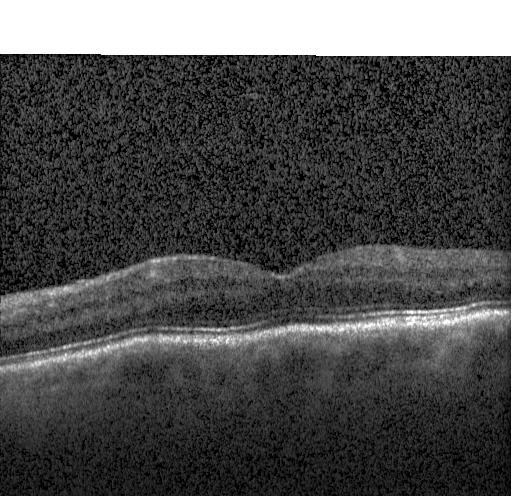
This B-scan demonstrates no CNV, no DME, and no drusen.